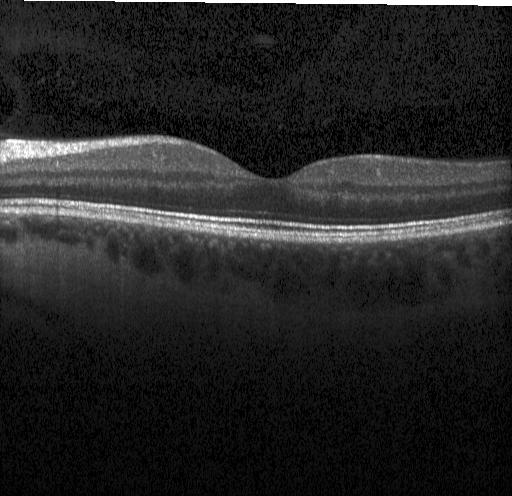

OCT line scan.
Impression: neither choroidal neovascularization, diabetic macular edema, nor drusen.